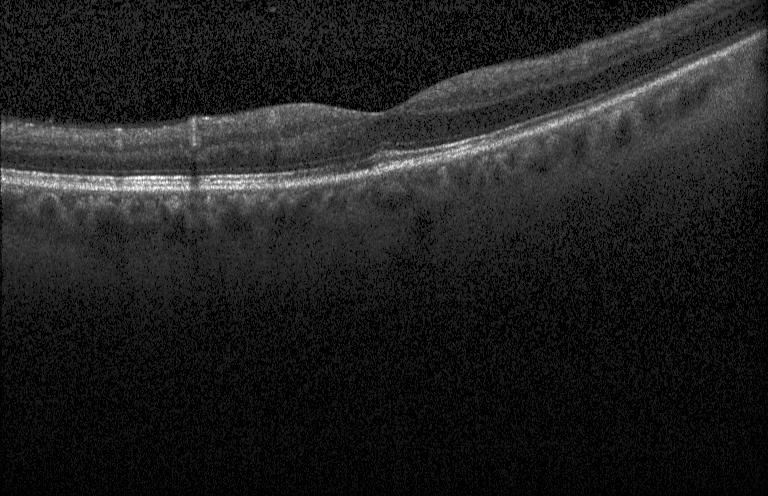 Macular OCT: neither CNV, DME, nor drusen.